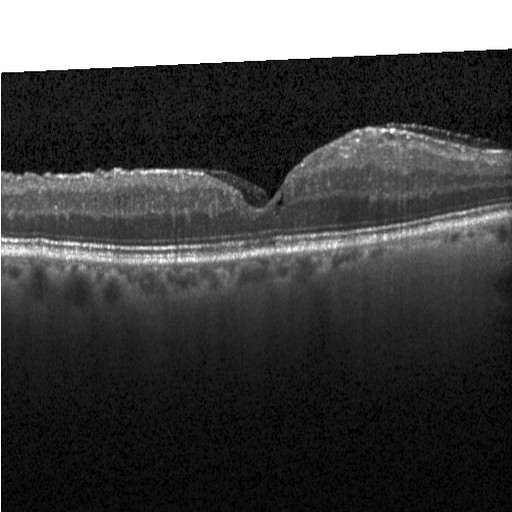

Fovea-centered; spectral-domain optical coherence tomography; OCT B-scan; Heidelberg Spectralis OCT system
Diabetic macular edema.